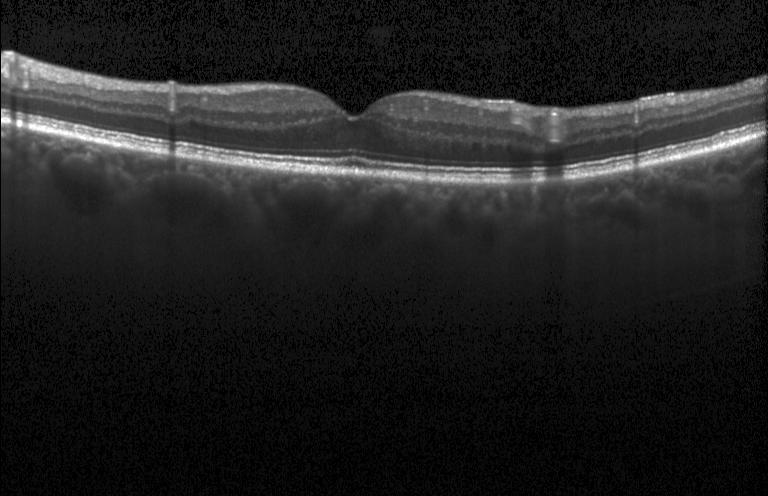
Optical coherence tomography B-scan, SD-OCT.
Neither CNV, DME, nor drusen.